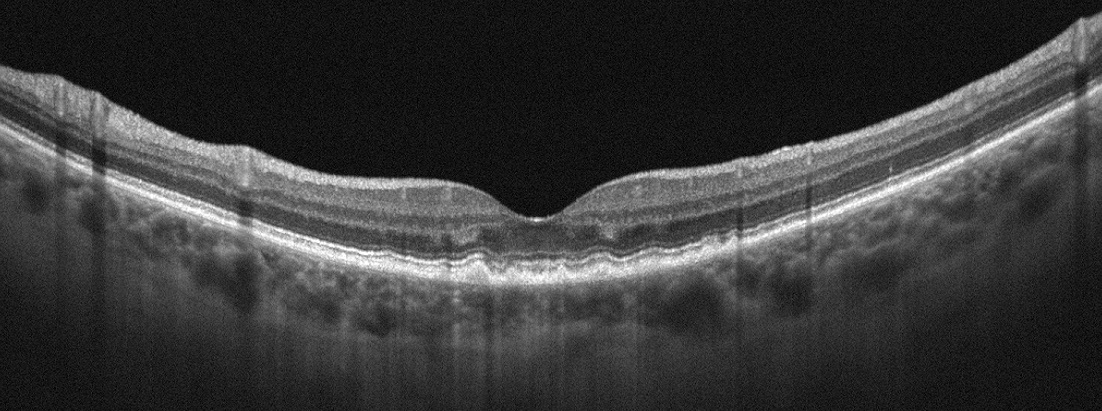
Macular scan; Optovue Avanti RTVue XR; retinal OCT B-scan.
Diagnosis: age-related macular degeneration.